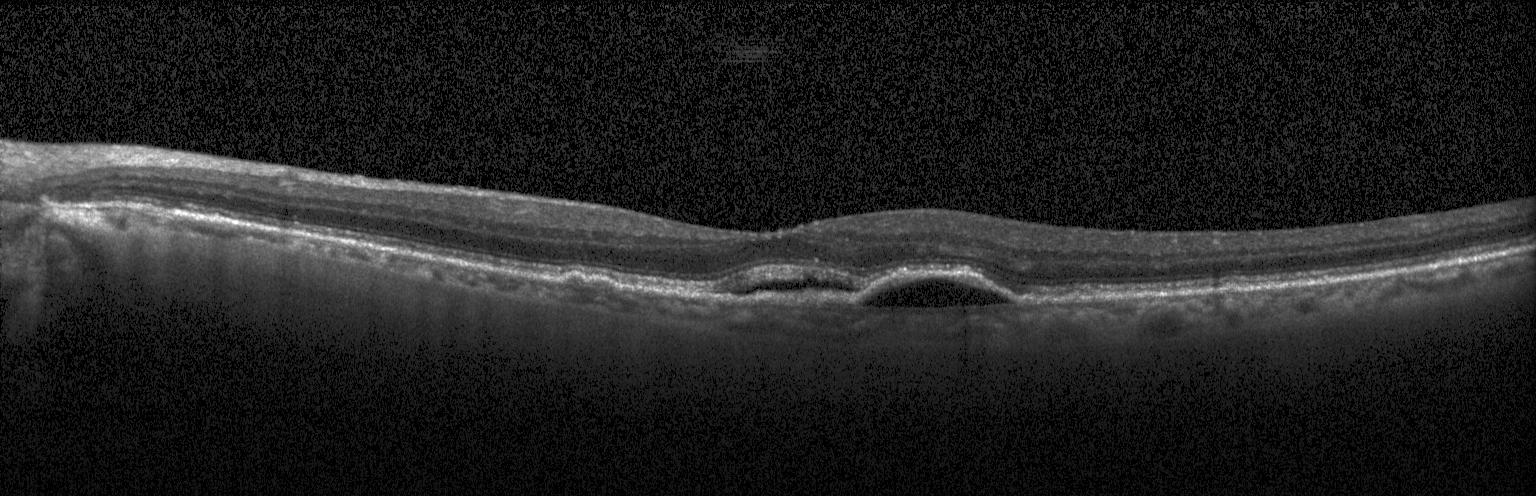 This B-scan demonstrates a choroidal neovascular membrane.